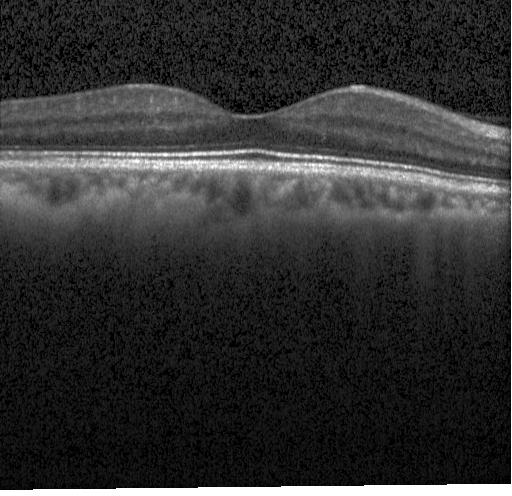

OCT line scan; macular scan — Dx: no evidence of choroidal neovascularization, diabetic macular edema, or drusen.